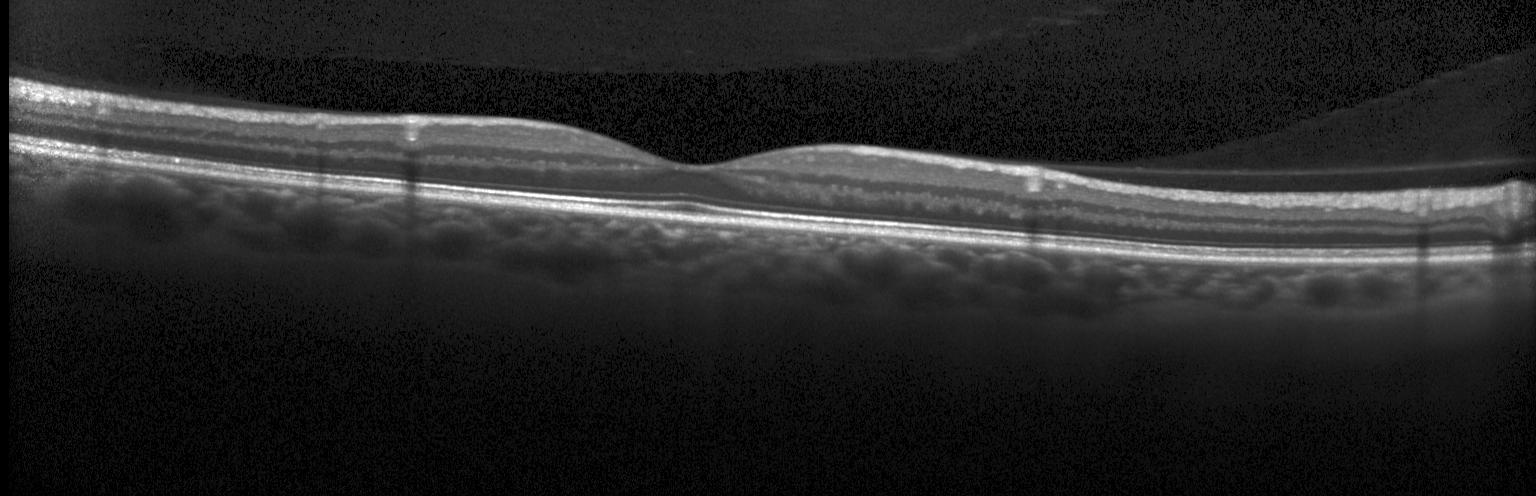
Macular scan; Heidelberg Spectralis OCT system; OCT B-scan.
Impression: neither CNV, DME, nor drusen.